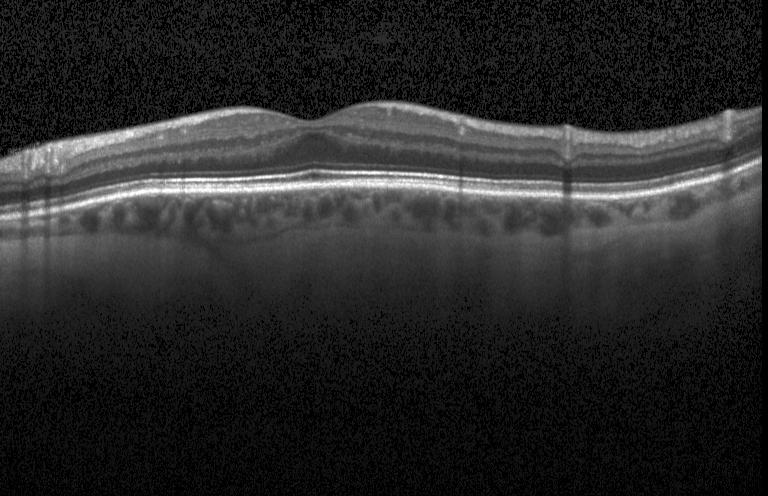

Through the macula · OCT line scan · Heidelberg Spectralis OCT system · SD-OCT.
Finding: no choroidal neovascularization, no diabetic macular edema, and no drusen.